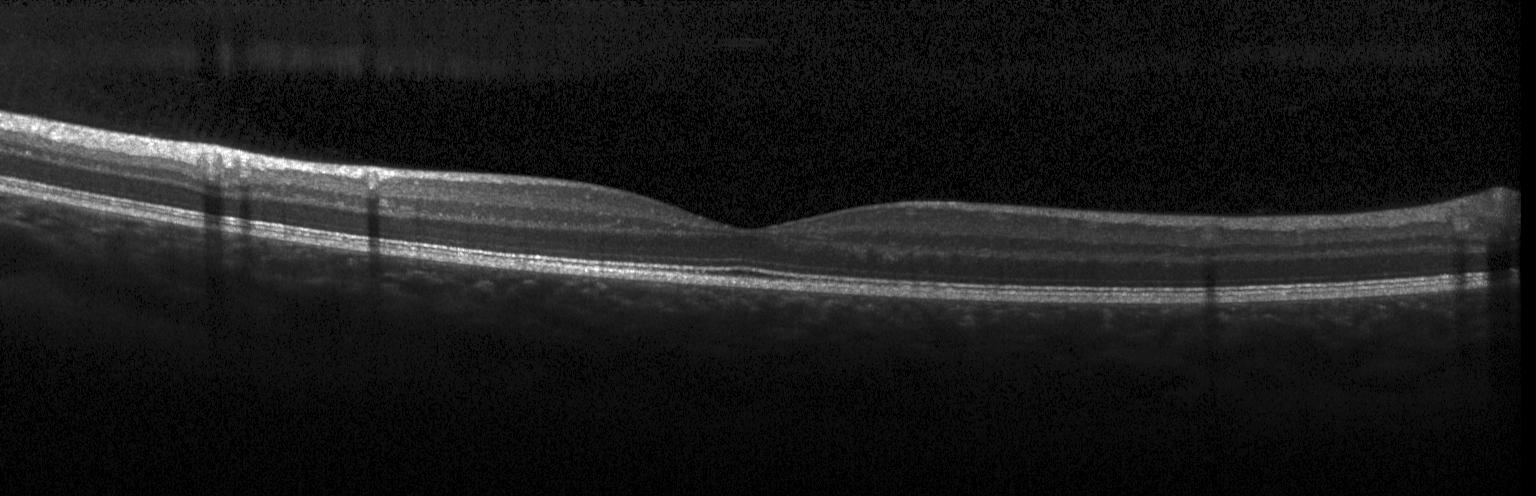

Optical coherence tomography scan · spectral-domain optical coherence tomography · Heidelberg Spectralis.
Diagnosis: neither CNV, DME, nor drusen.